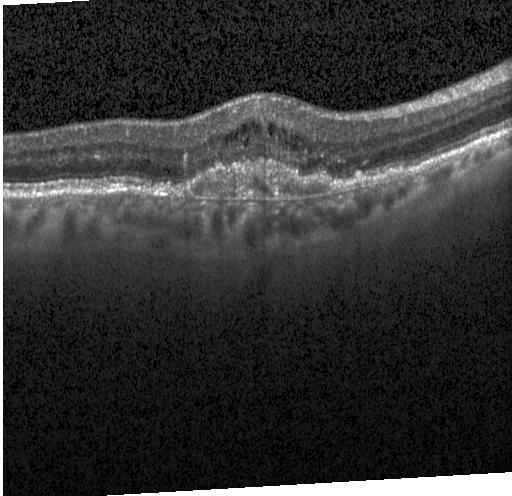
Fovea-centered, acquired on a Heidelberg Spectralis, optical coherence tomography scan.
Finding: CNV.